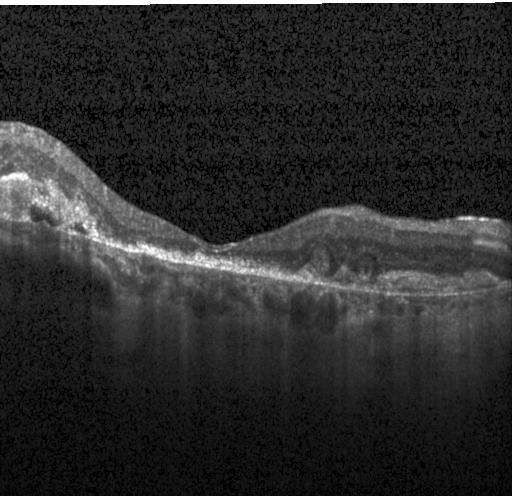 Finding: a choroidal neovascular membrane.